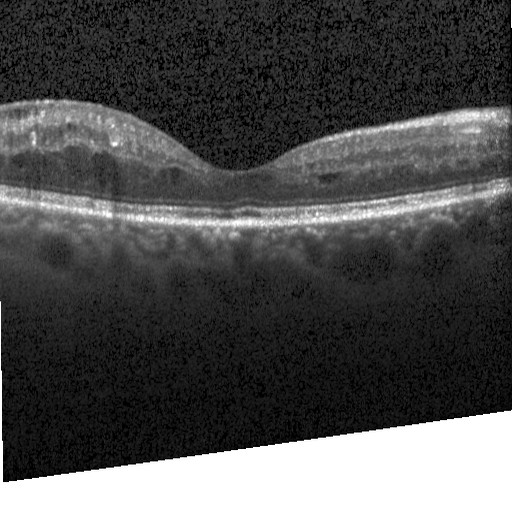

Fovea-centered; SD-OCT; OCT B-scan — Dx: diabetic macular edema (DME).